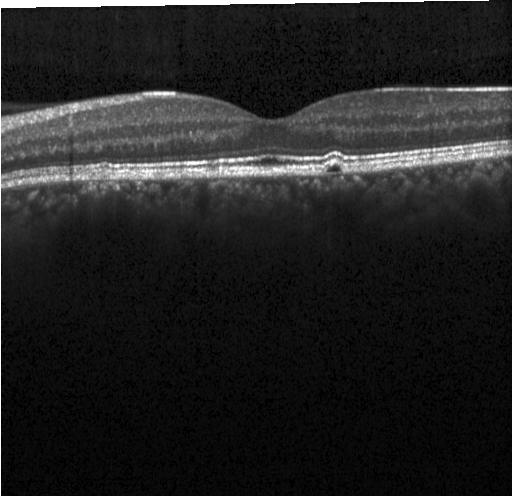

Optical coherence tomography scan. Macular OCT: drusen.